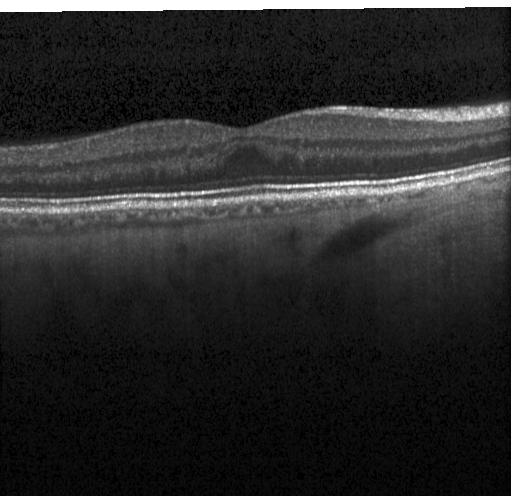
Instrument: Heidelberg Spectralis, retinal OCT B-scan — Diagnosis: no CNV, no DME, and no drusen.